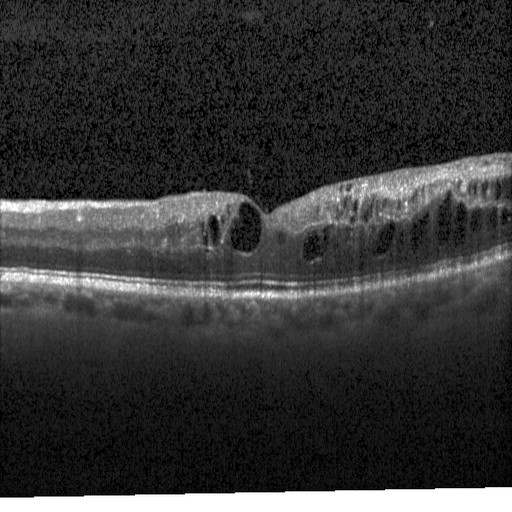
Spectral-domain OCT B-scan: diabetic macular edema.